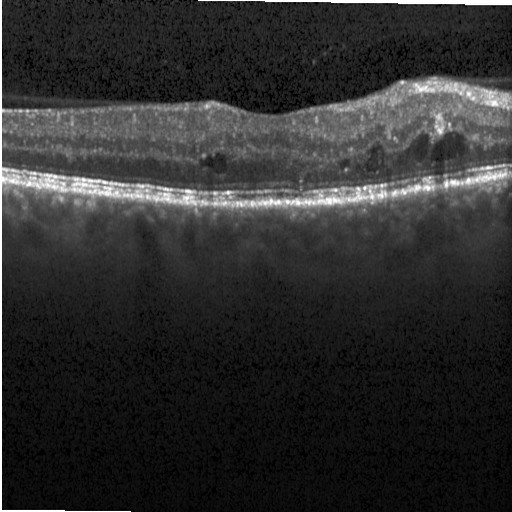
Impression: DME.